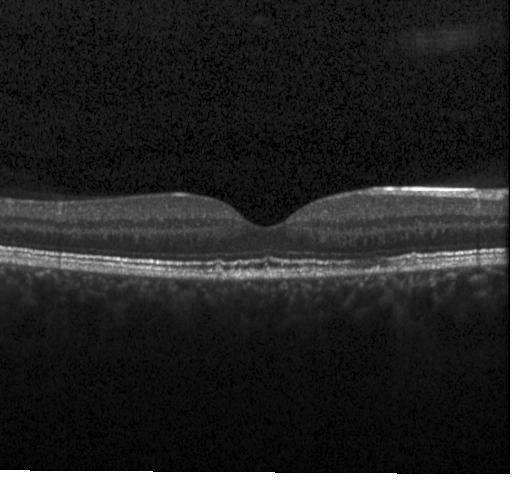
Finding: multiple drusen.